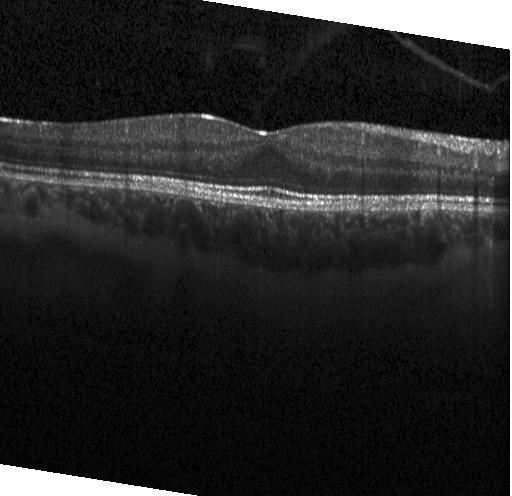 Horizontal scan through the fovea, instrument: Heidelberg Spectralis, spectral-domain OCT, optical coherence tomography B-scan.
Impression: no choroidal neovascularization, diabetic macular edema, or drusen.